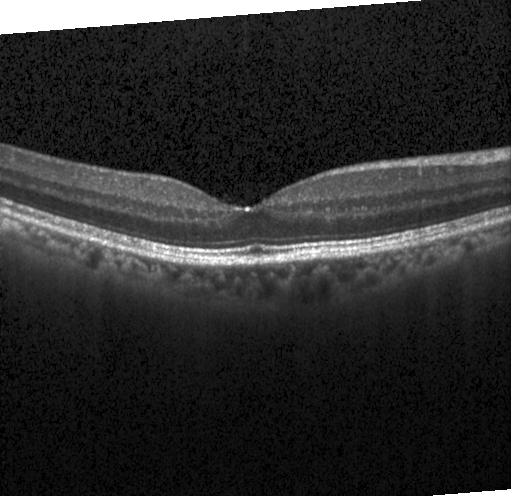 Retinal OCT B-scan
Impression: no choroidal neovascularization, no diabetic macular edema, and no drusen.